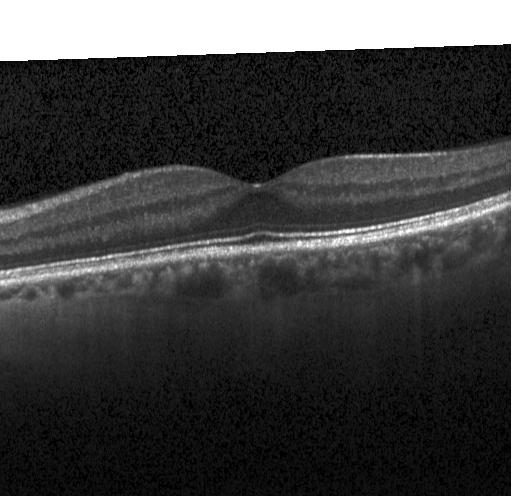
Spectral-domain optical coherence tomography. OCT line scan. Heidelberg Spectralis OCT system. Fovea-centered — The scan shows neither CNV, DME, nor drusen.